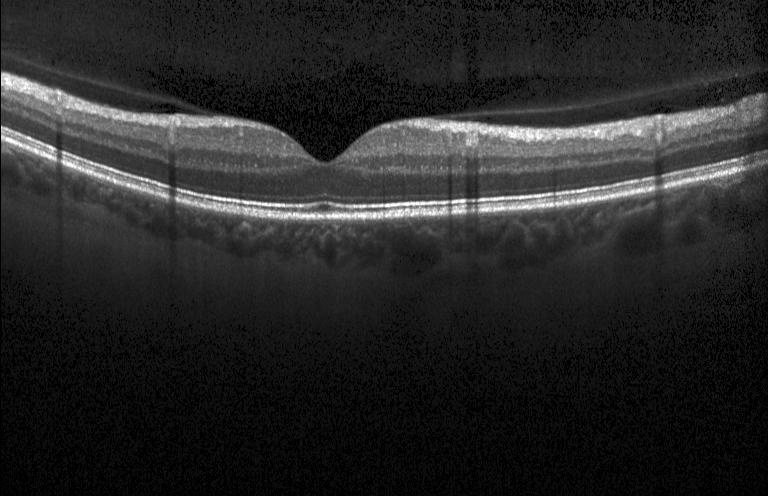 No CNV, no DME, and no drusen.